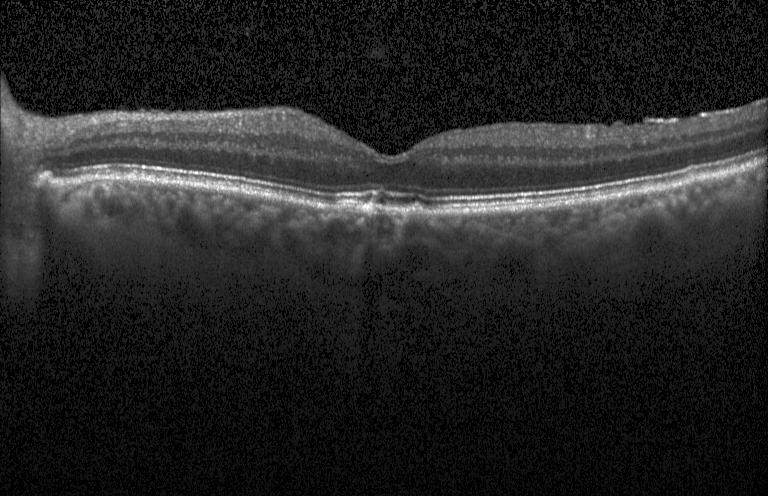

Acquired on a Heidelberg Spectralis, optical coherence tomography B-scan, horizontal scan through the fovea
Multiple drusen.